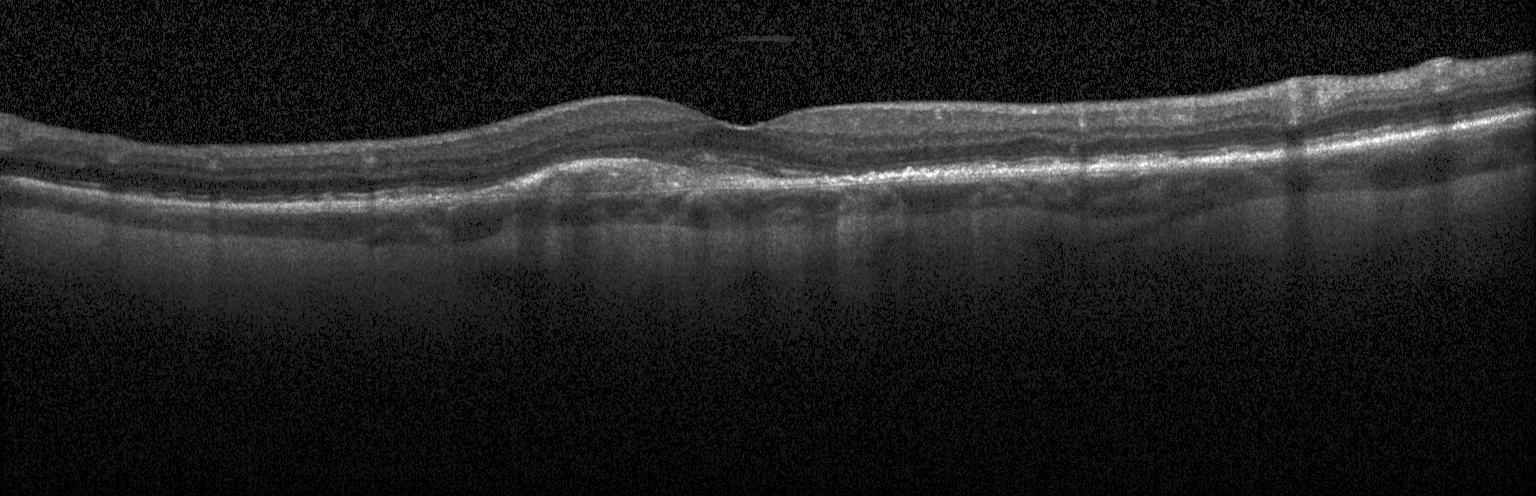 SD-OCT, optical coherence tomography B-scan, acquired on a Heidelberg Spectralis. Impression: a choroidal neovascular membrane.